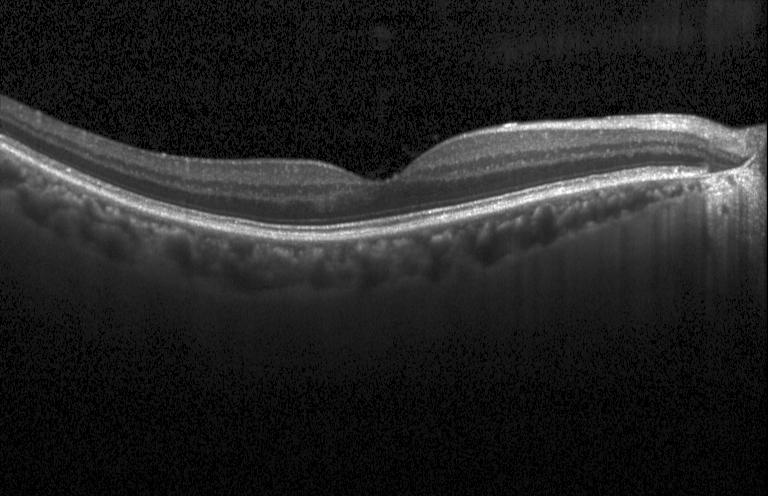
Through the macula, retinal OCT cross-section — Impression: neither choroidal neovascularization, diabetic macular edema, nor drusen.